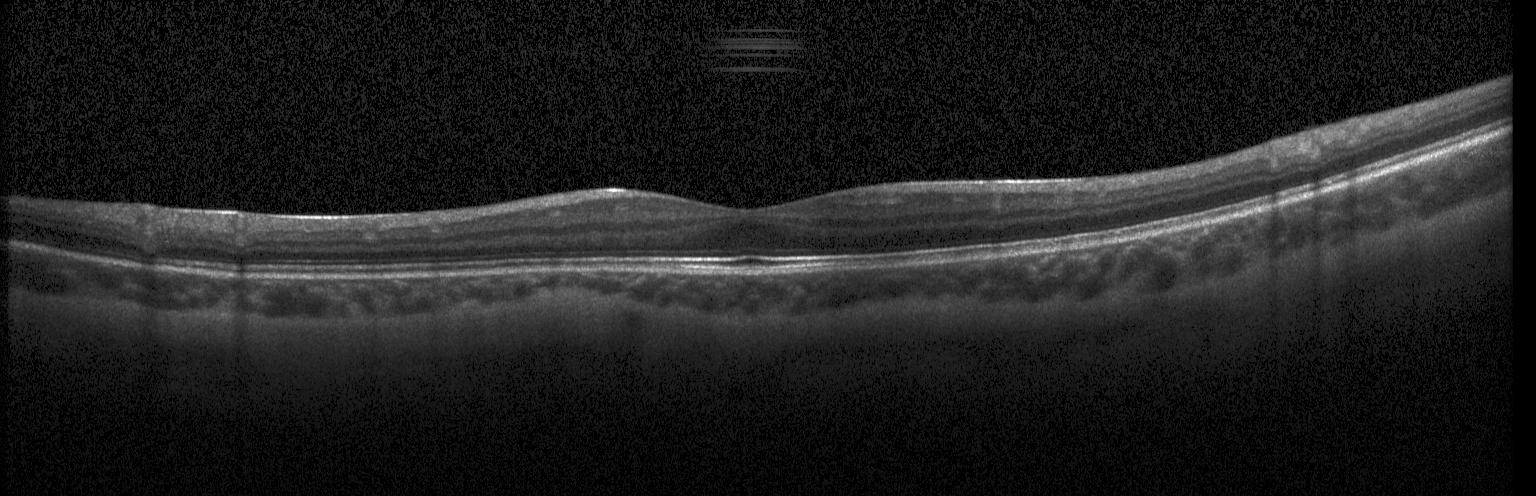
Impression: no evidence of CNV, DME, or drusen.